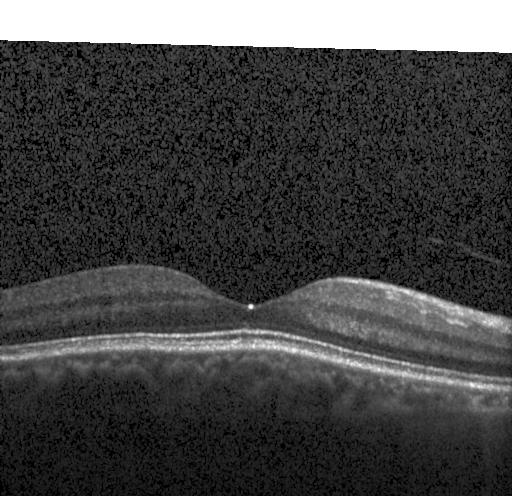 OCT finding: no evidence of choroidal neovascularization, diabetic macular edema, or drusen.